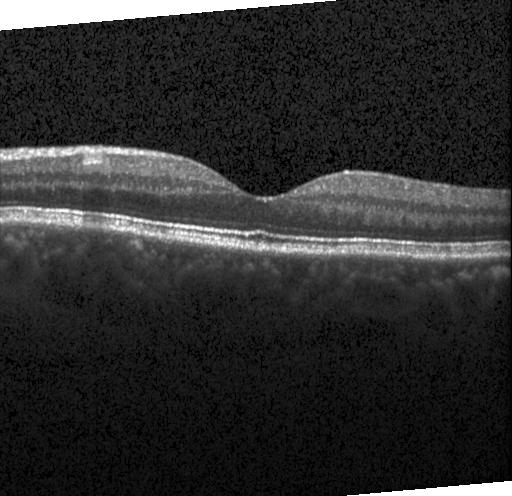

Optical coherence tomography B-scan, SD-OCT — This B-scan demonstrates neither choroidal neovascularization, diabetic macular edema, nor drusen.